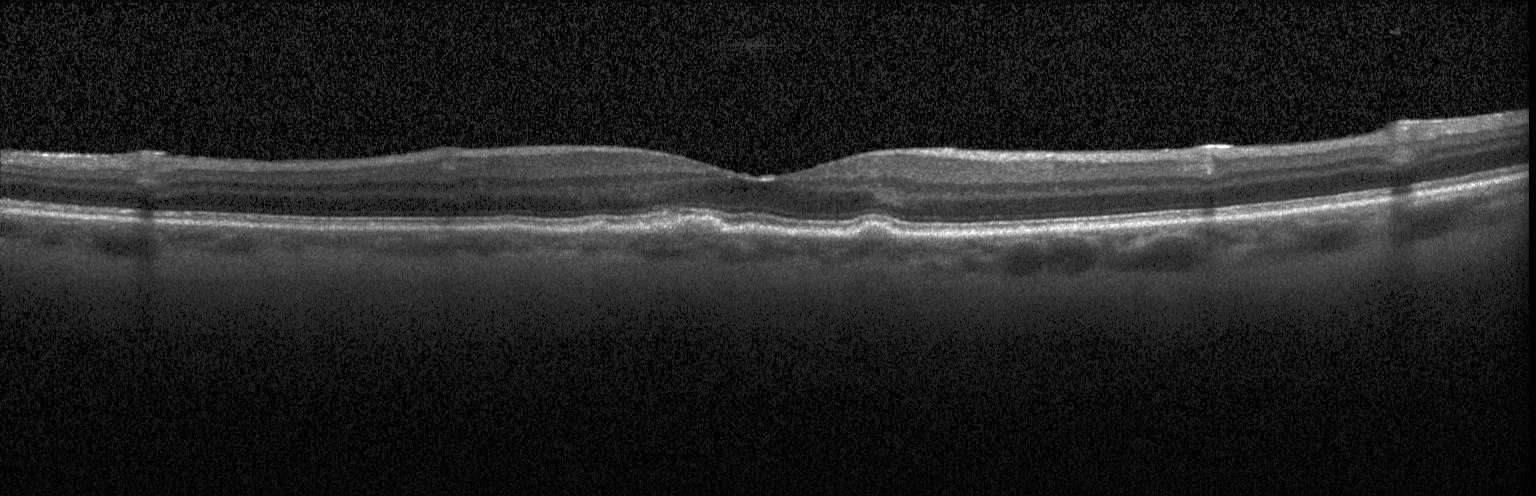

Optical coherence tomography B-scan · instrument: Heidelberg Spectralis — The scan shows multiple drusen.